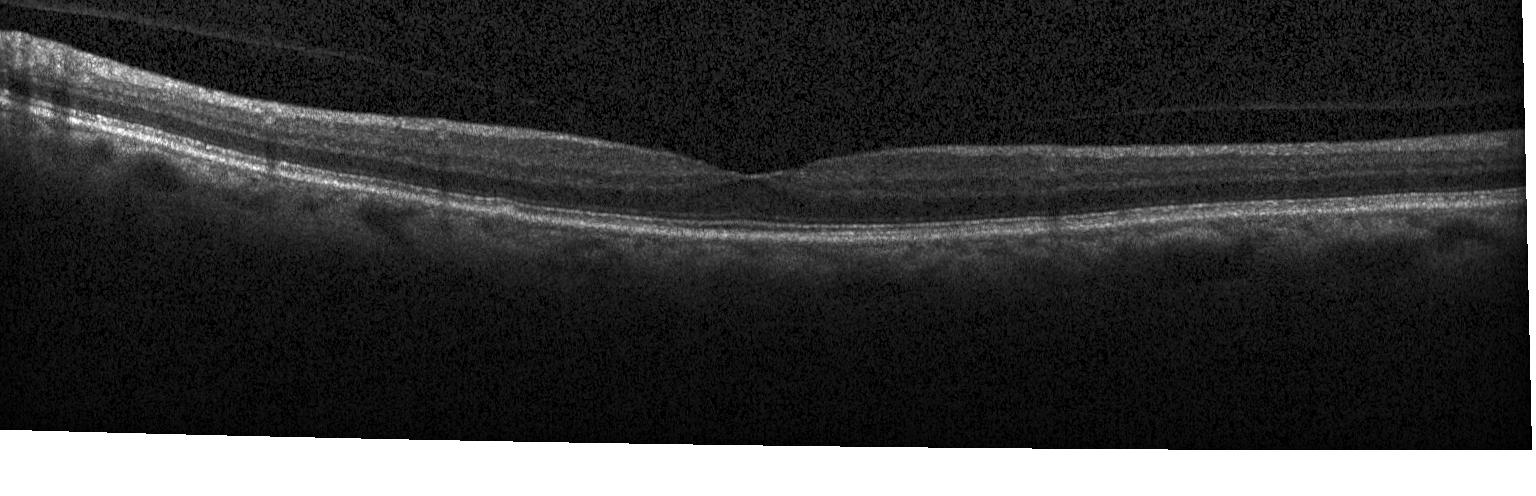
OCT B-scan · horizontal scan through the fovea · spectral-domain OCT · Heidelberg Spectralis OCT system
Finding: no evidence of CNV, DME, or drusen.